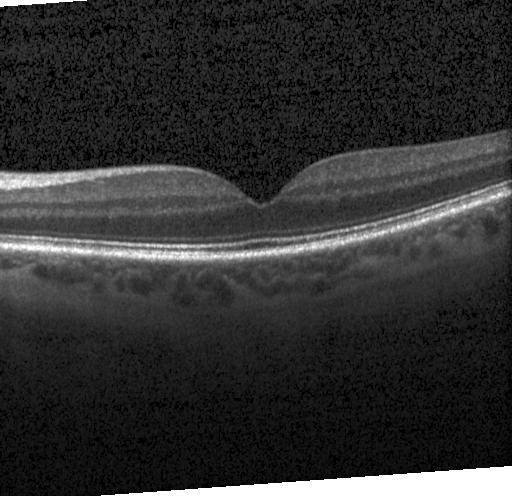

OCT line scan
Dx: neither choroidal neovascularization, diabetic macular edema, nor drusen.